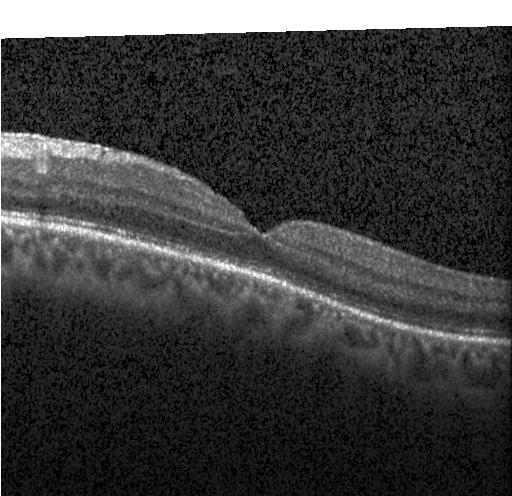 OCT B-scan
OCT finding: no choroidal neovascularization, no diabetic macular edema, and no drusen.